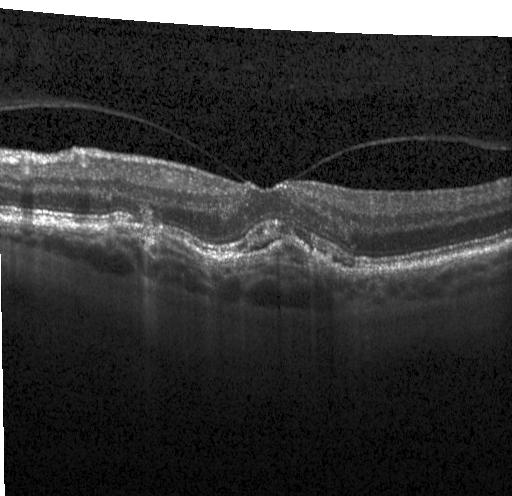
OCT line scan. Spectral-domain optical coherence tomography. Assessment: CNV.